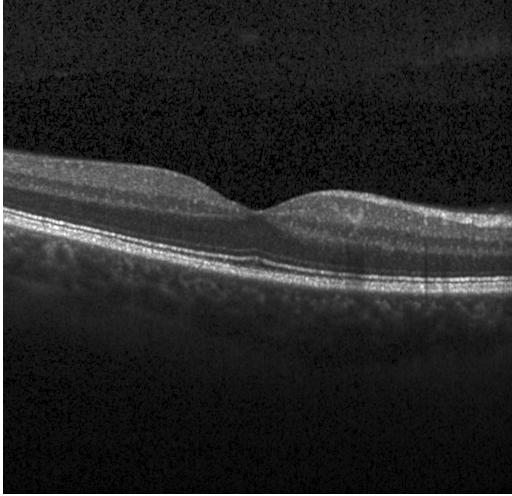

OCT line scan; spectral-domain optical coherence tomography — Finding: no choroidal neovascularization, diabetic macular edema, or drusen.